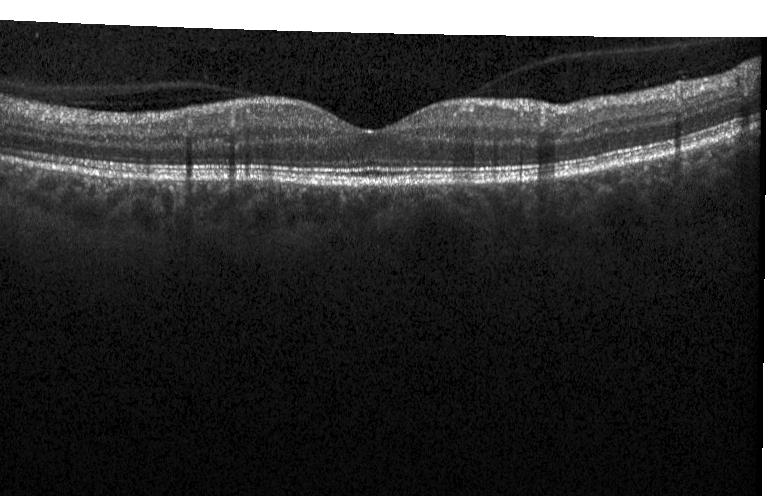 OCT scan showing neither choroidal neovascularization, diabetic macular edema, nor drusen.